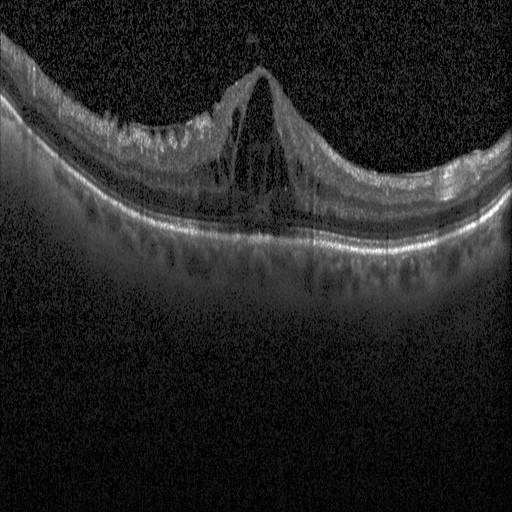

Diagnosis: DME.